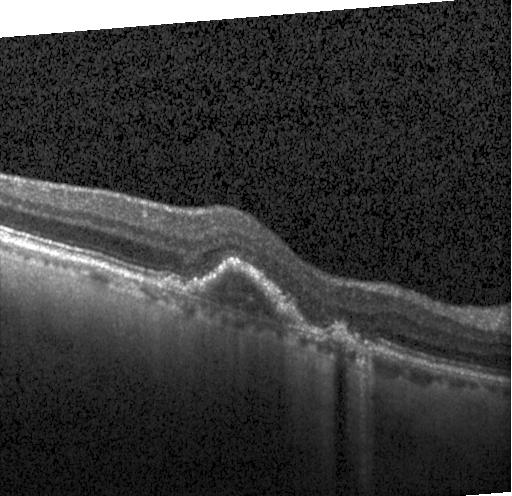

Macular scan · retinal OCT B-scan — Finding: a choroidal neovascular membrane.